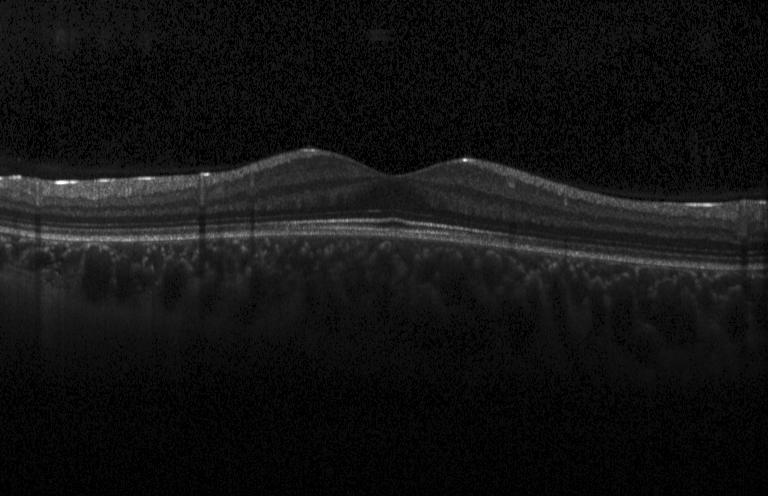

OCT finding: no evidence of choroidal neovascularization, diabetic macular edema, or drusen.